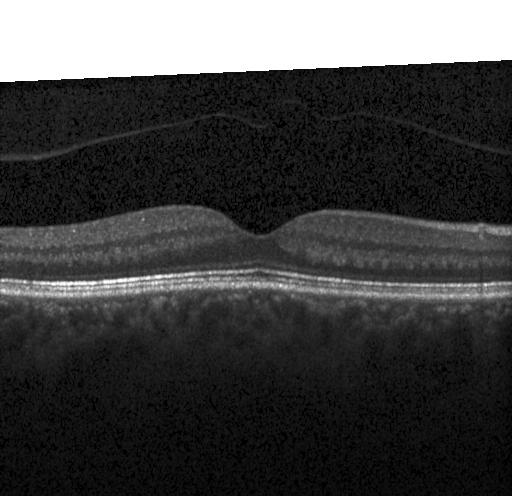
SD-OCT. Heidelberg Spectralis. Horizontal scan through the fovea. OCT line scan
Dx: no choroidal neovascularization, diabetic macular edema, or drusen.